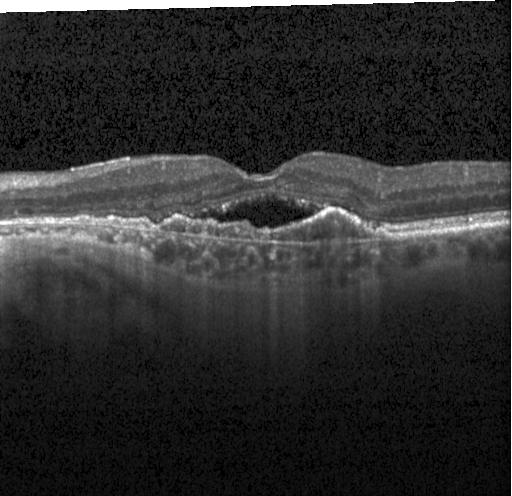

Macular OCT: choroidal neovascularization (CNV).